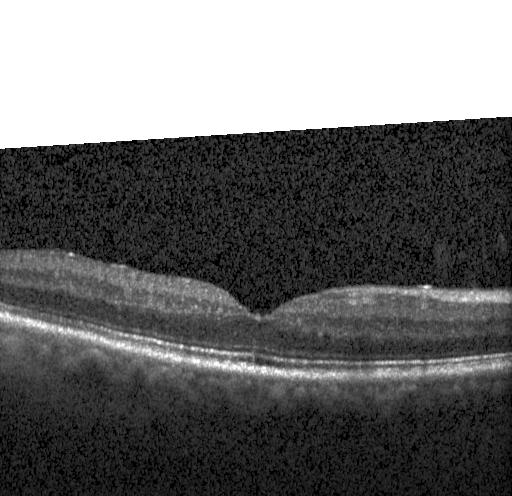 Acquired on a Heidelberg Spectralis, OCT line scan, macular scan, spectral-domain OCT
This B-scan demonstrates no evidence of CNV, DME, or drusen.